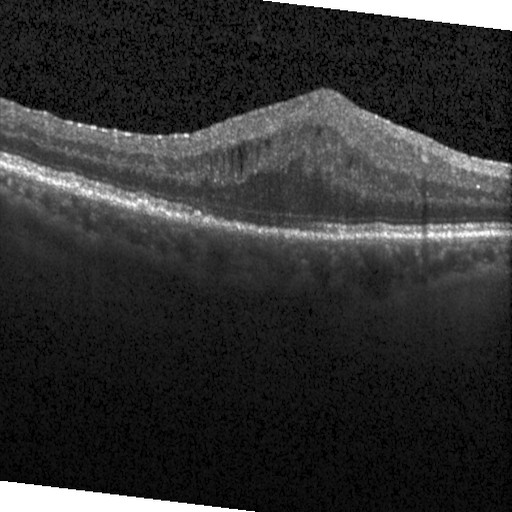 Heidelberg Spectralis · spectral-domain optical coherence tomography · OCT line scan. Impression: DME.